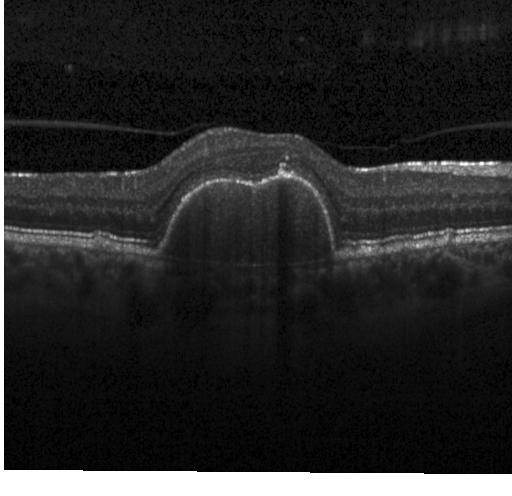

Macular OCT: a choroidal neovascular membrane.